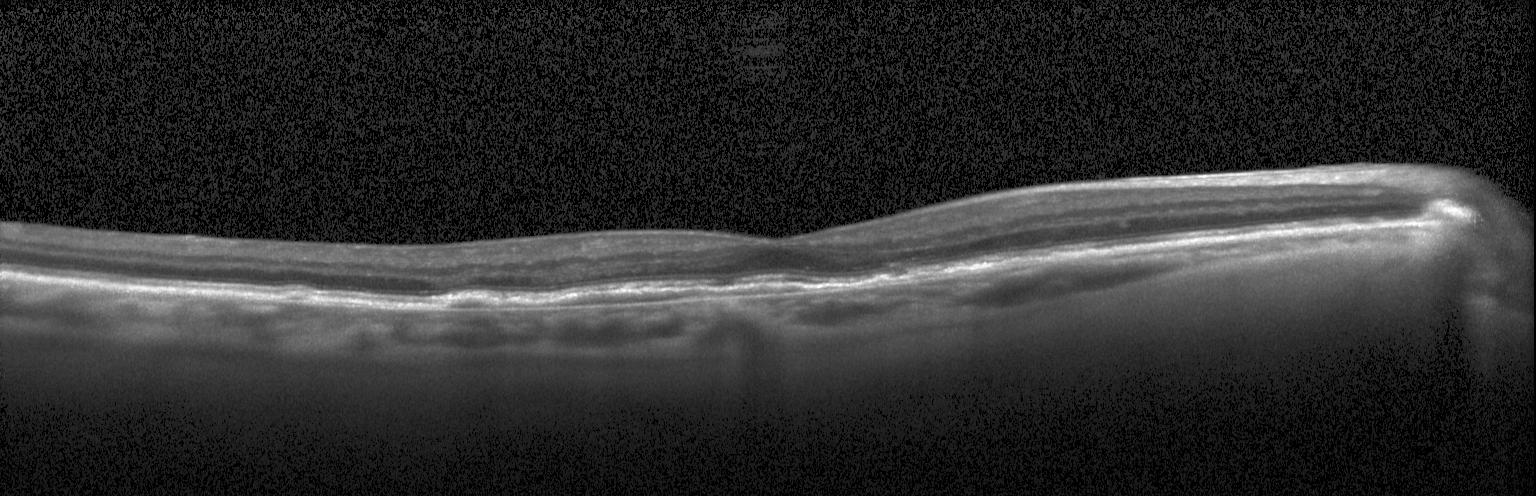
Spectral-domain OCT B-scan: a choroidal neovascular membrane.